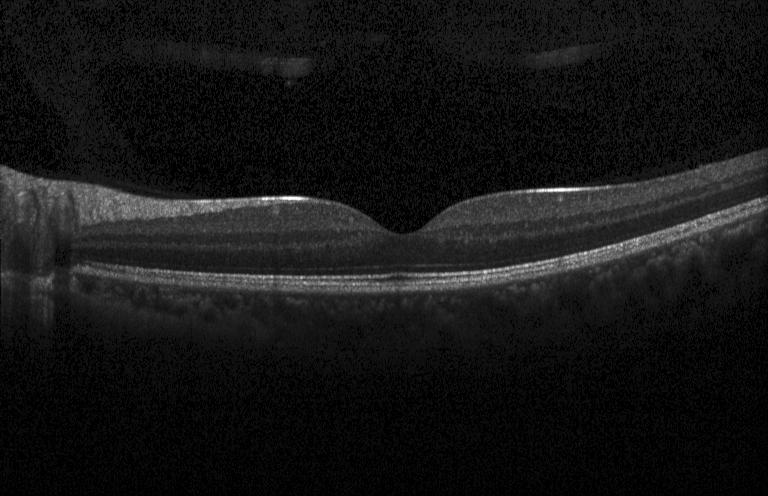

Neither choroidal neovascularization, diabetic macular edema, nor drusen.